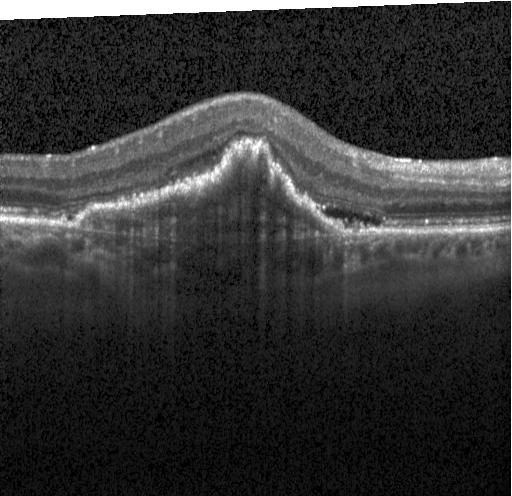

The scan shows choroidal neovascularization.